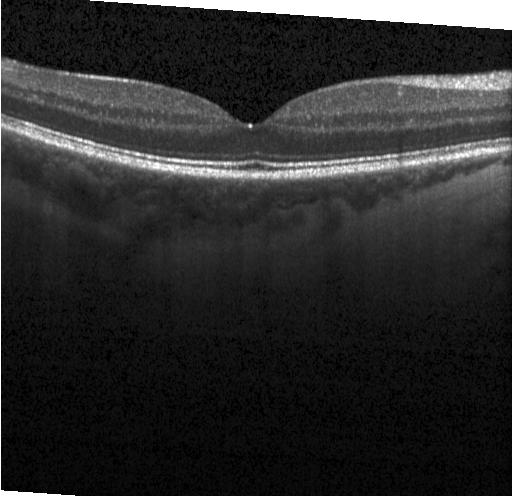

Instrument: Heidelberg Spectralis, optical coherence tomography B-scan
Dx: neither choroidal neovascularization, diabetic macular edema, nor drusen.